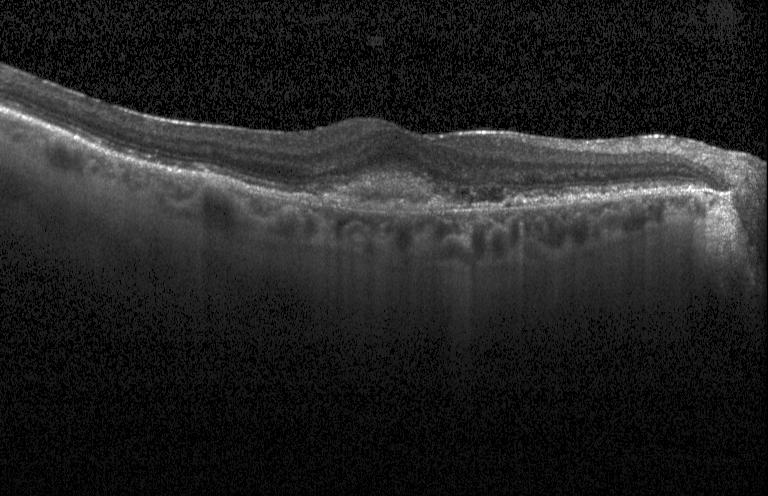

Spectral-domain OCT. Optical coherence tomography scan. Heidelberg Spectralis. Through the macula — Dx: a choroidal neovascular membrane.